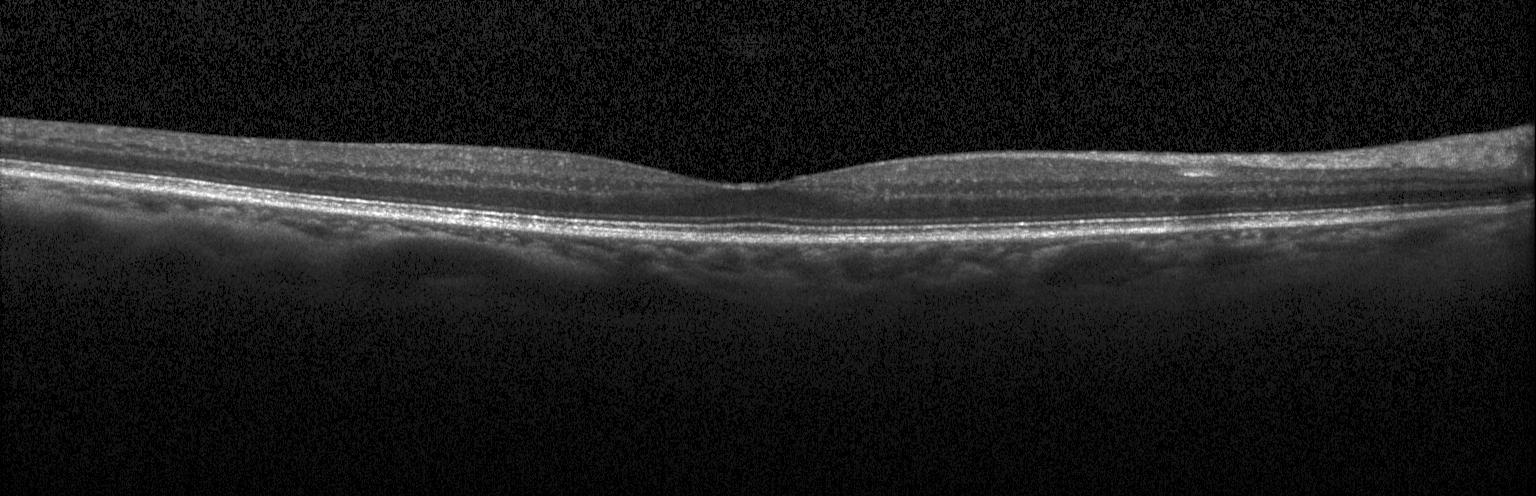 OCT line scan; fovea-centered. The scan shows no evidence of choroidal neovascularization, diabetic macular edema, or drusen.